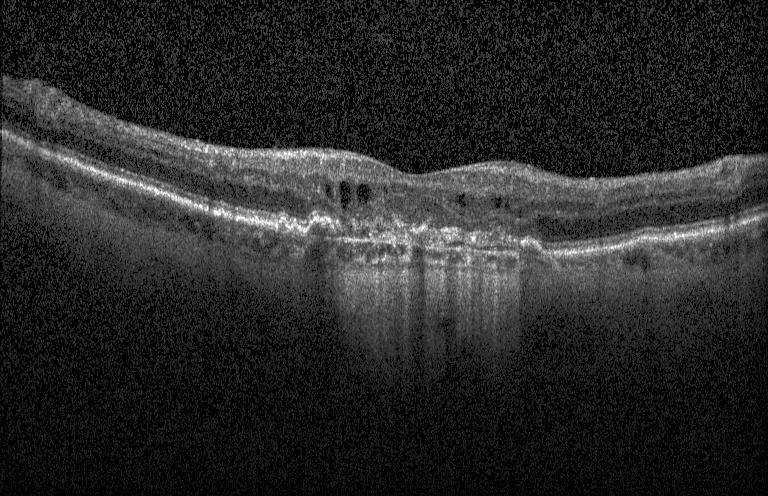

OCT line scan — This B-scan demonstrates a choroidal neovascular membrane.